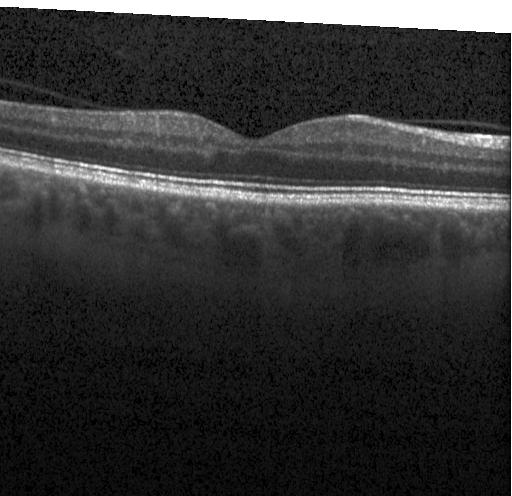

SD-OCT. Centered on the fovea. OCT B-scan. Instrument: Heidelberg Spectralis.
Finding: no CNV, no DME, and no drusen.